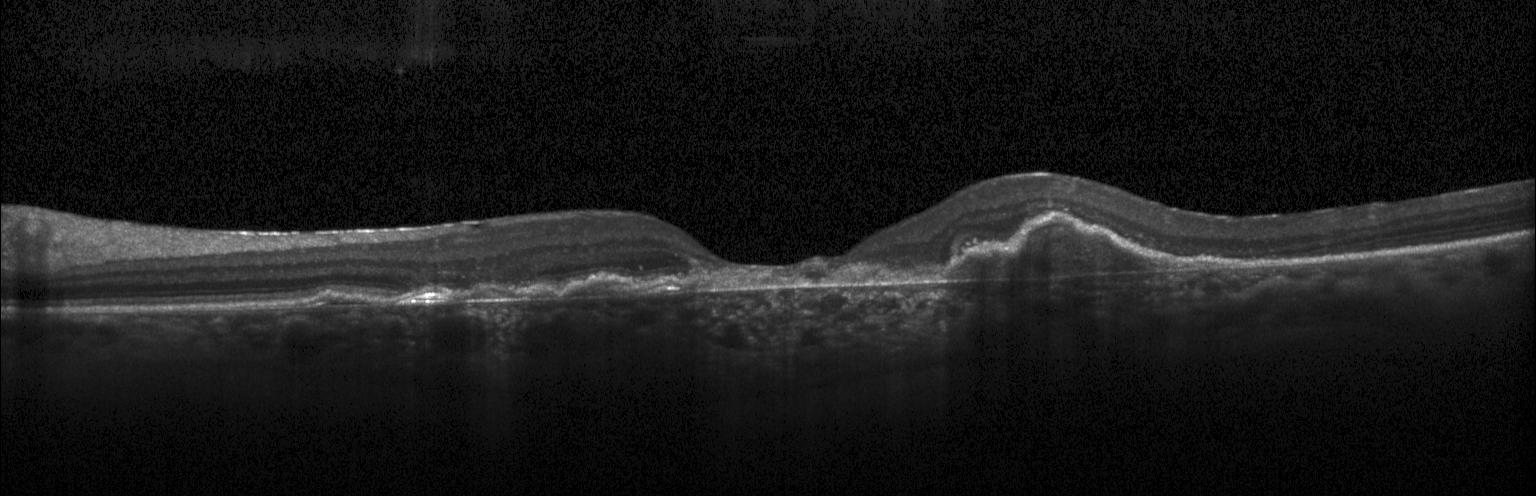 SD-OCT; fovea-centered; retinal OCT B-scan. Dx: choroidal neovascularization.